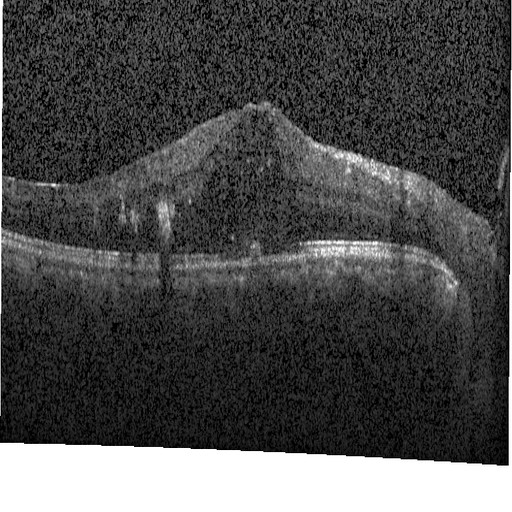

Retinal OCT cross-section; horizontal scan through the fovea; instrument: Heidelberg Spectralis.
Impression: diabetic macular edema.